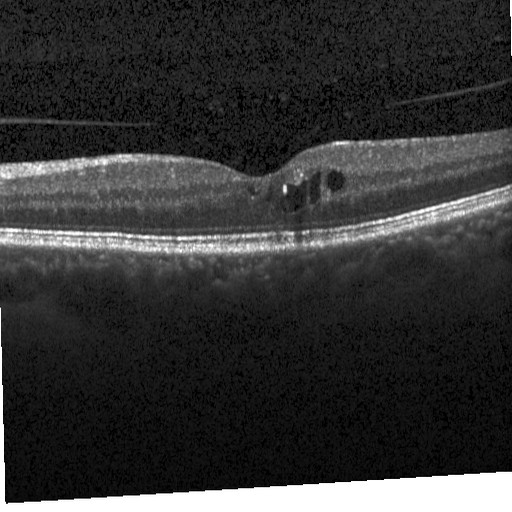
Impression: diabetic macular edema.